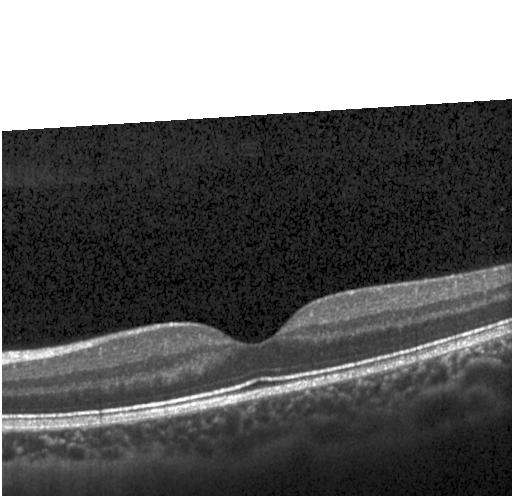
No CNV, DME, or drusen.